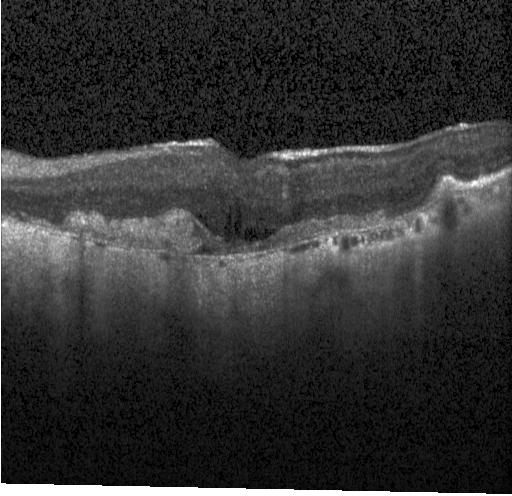

Diagnosis: a choroidal neovascular membrane.